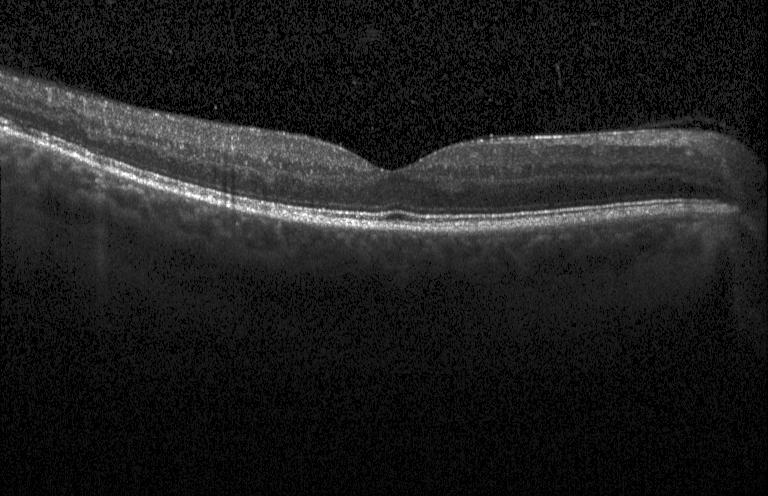
OCT line scan — Assessment: no choroidal neovascularization, diabetic macular edema, or drusen.